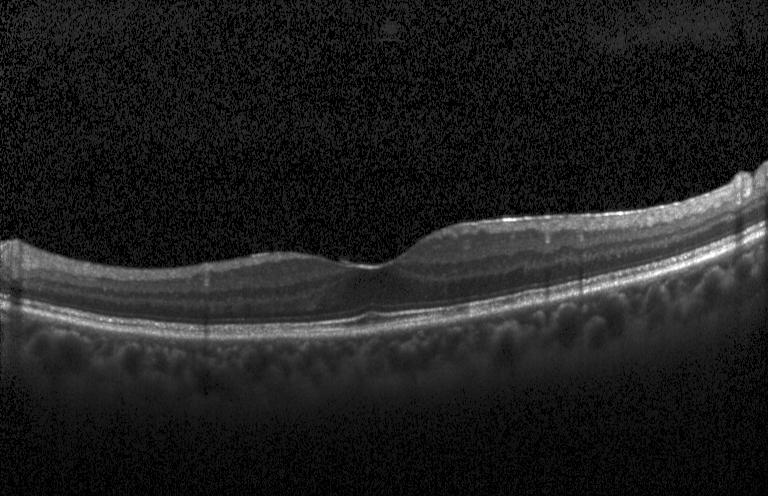 OCT line scan; SD-OCT — Diagnosis: no evidence of CNV, DME, or drusen.